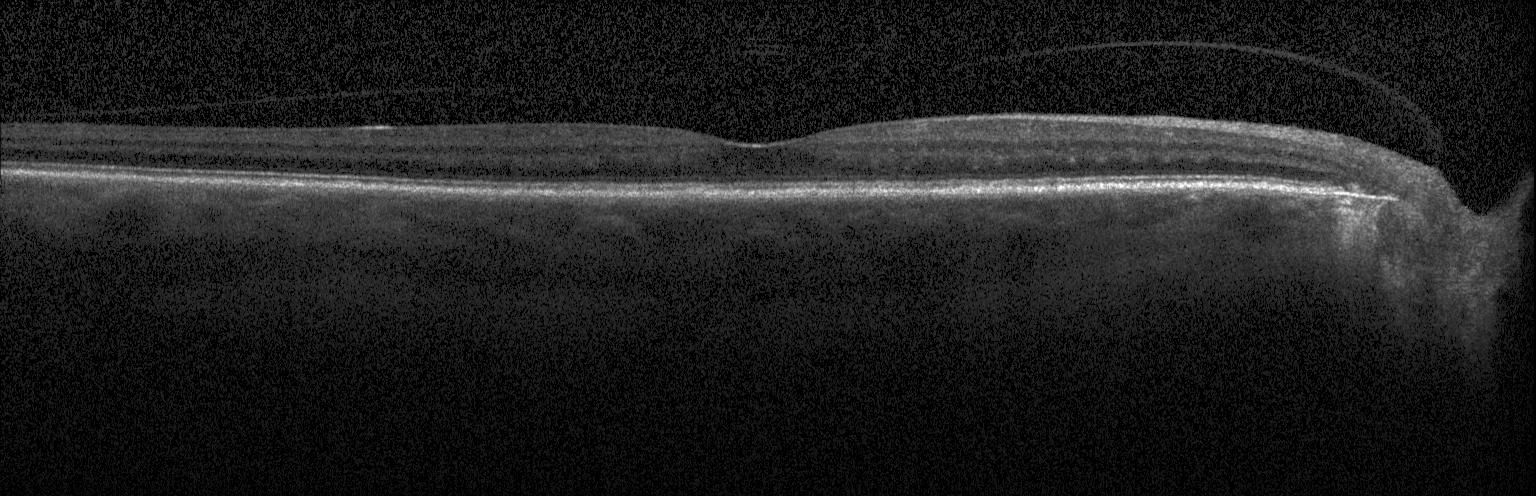 OCT scan showing neither choroidal neovascularization, diabetic macular edema, nor drusen.